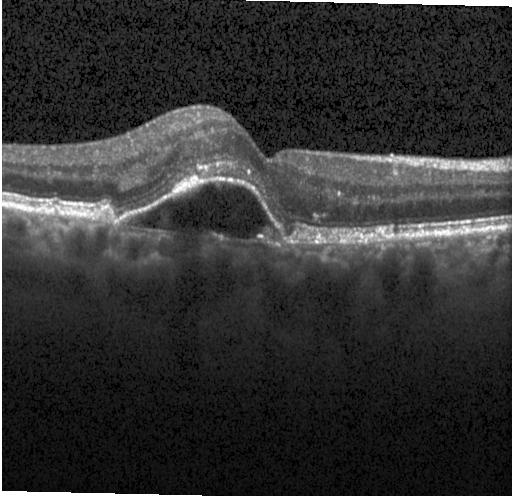 Heidelberg Spectralis; retinal OCT B-scan; through the macula; spectral-domain optical coherence tomography.
The scan shows choroidal neovascularization (CNV).